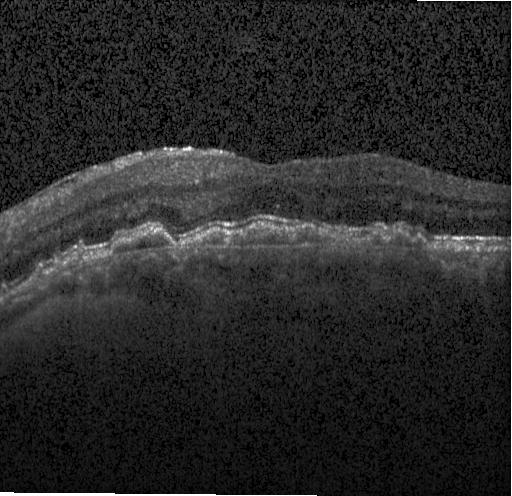 Macular OCT: a choroidal neovascular membrane.